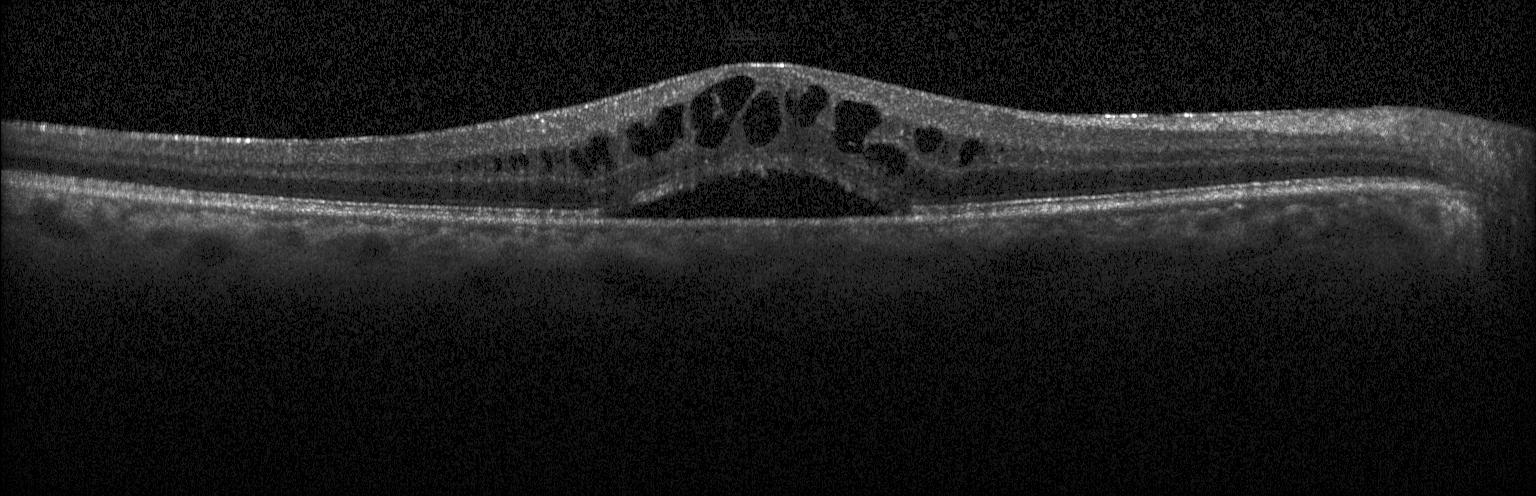
Spectral-domain optical coherence tomography; retinal OCT cross-section; instrument: Heidelberg Spectralis
Assessment: diabetic macular edema.